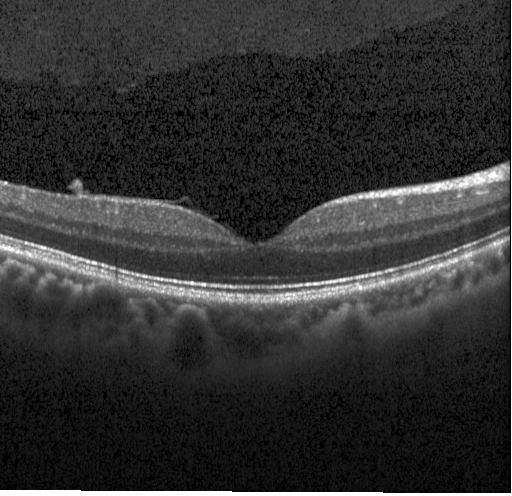

OCT scan showing no CNV, DME, or drusen.